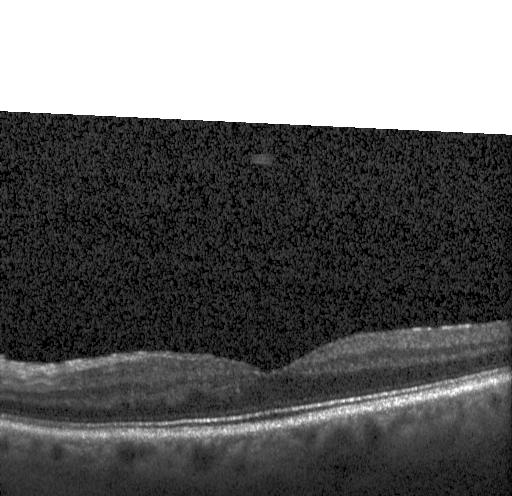
Diagnosis: no evidence of CNV, DME, or drusen.